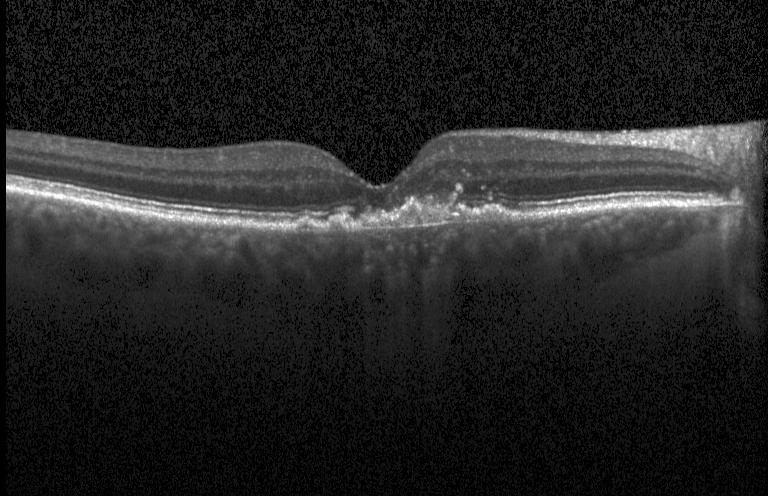 Optical coherence tomography B-scan · fovea-centered · Heidelberg Spectralis · spectral-domain OCT. A choroidal neovascular membrane.